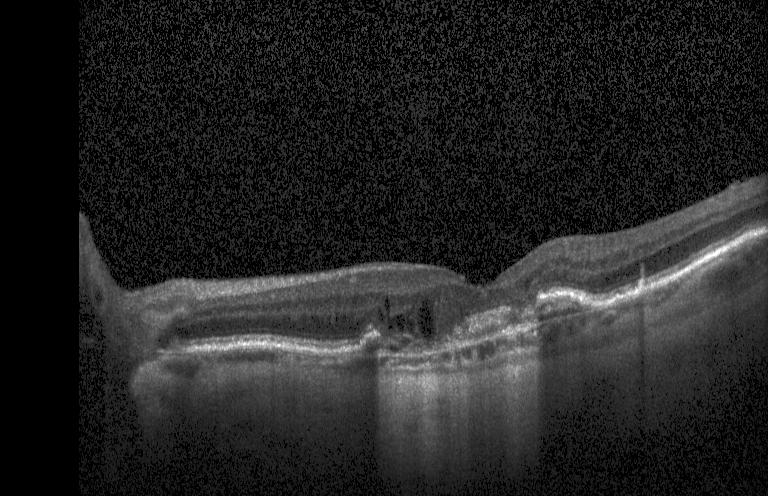 OCT line scan · spectral-domain OCT · Heidelberg Spectralis · macular scan
The scan shows a choroidal neovascular membrane.